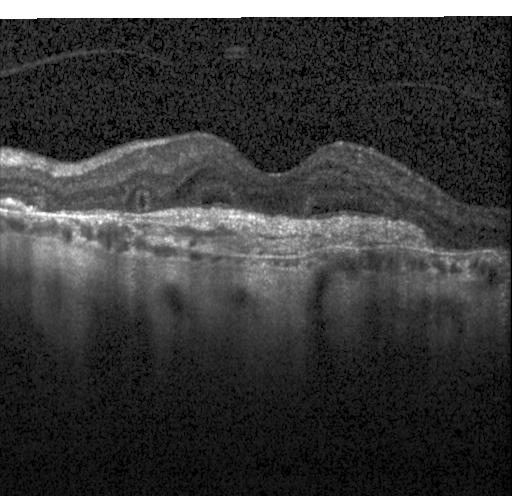
Finding: a choroidal neovascular membrane.